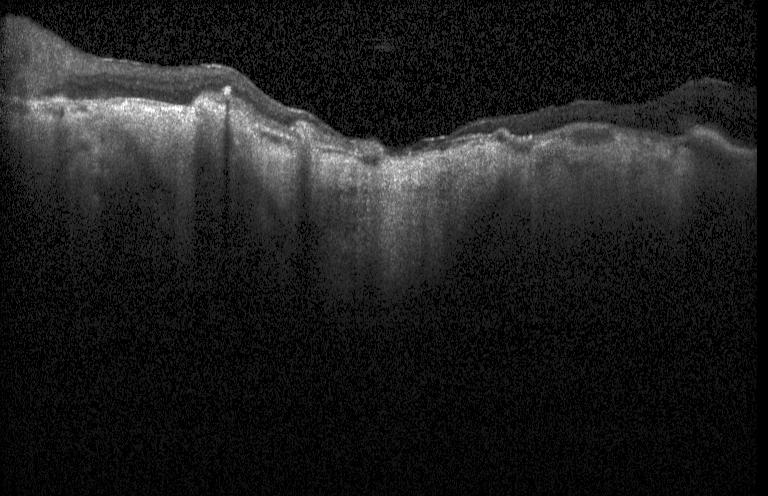
OCT scan showing a choroidal neovascular membrane.